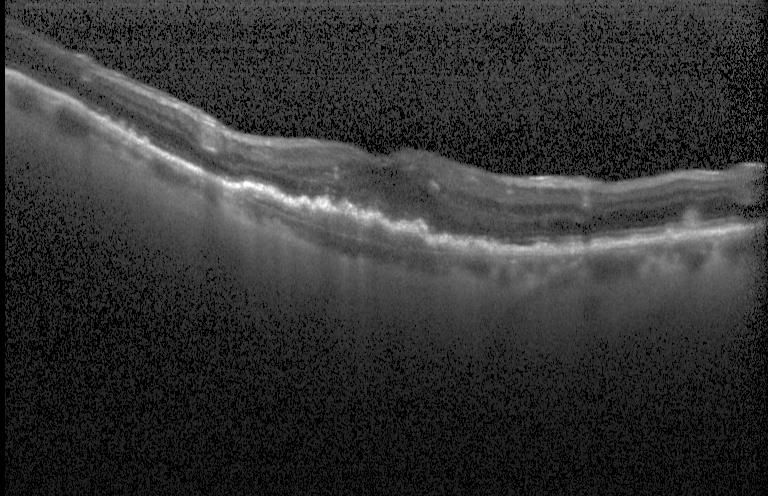 Finding: choroidal neovascularization (CNV).